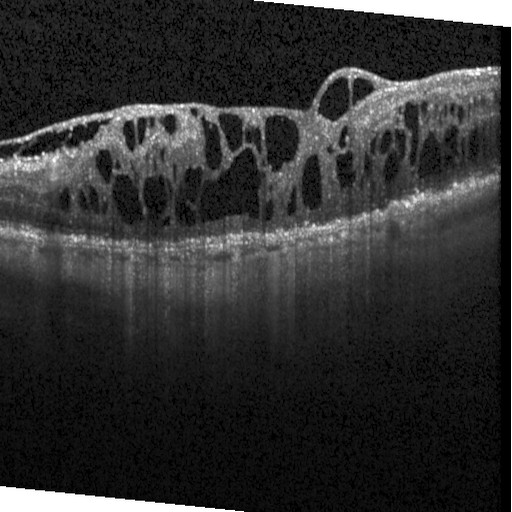 The scan shows diabetic macular edema (DME).